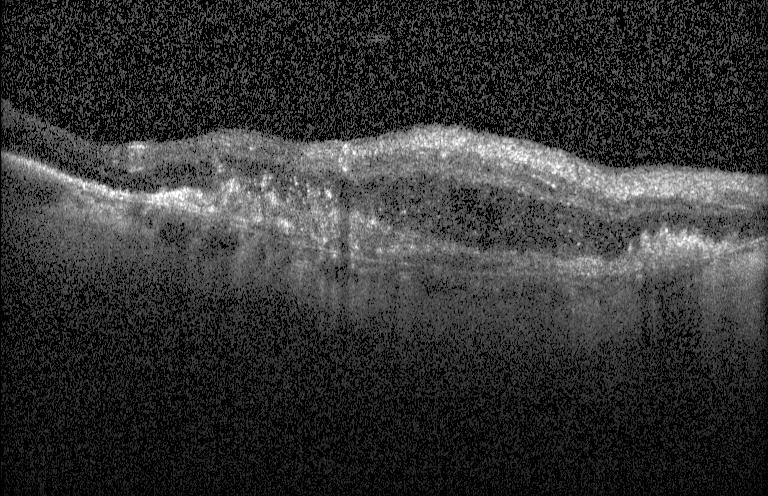

Optical coherence tomography B-scan. Diagnosis: CNV.